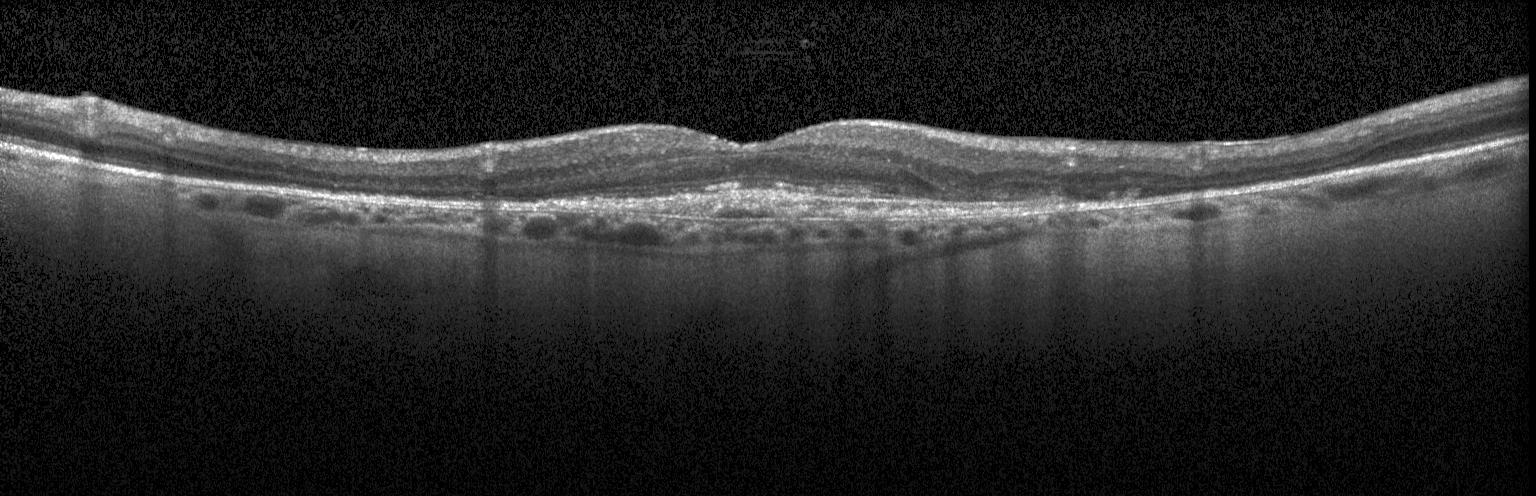
Retinal OCT cross-section showing choroidal neovascularization.